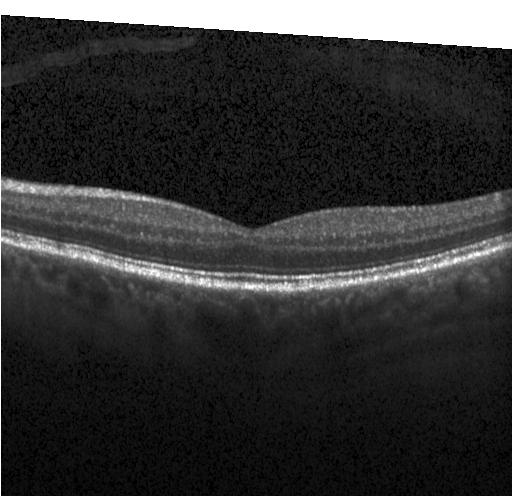
Acquired on a Heidelberg Spectralis; optical coherence tomography B-scan
Macular OCT: no choroidal neovascularization, no diabetic macular edema, and no drusen.